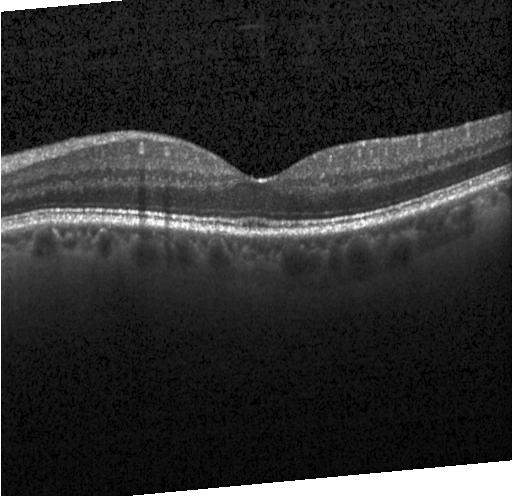

OCT finding: no choroidal neovascularization, no diabetic macular edema, and no drusen.